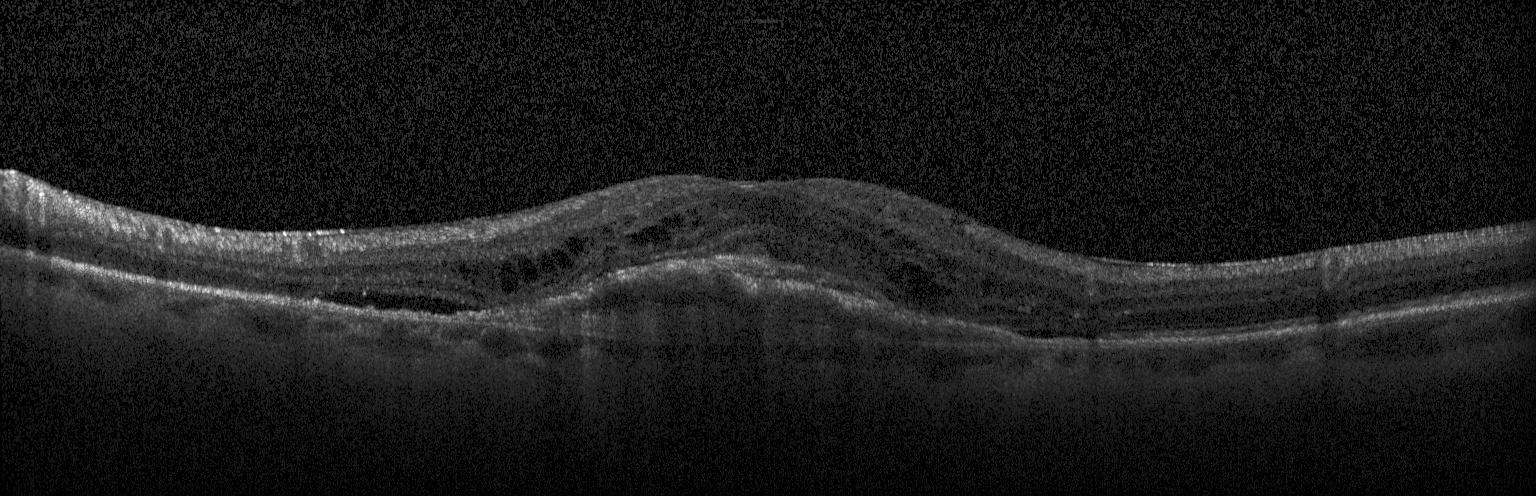
Macular OCT: a choroidal neovascular membrane.